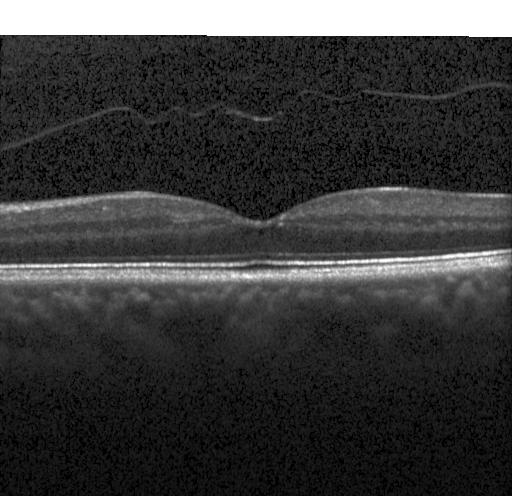 Horizontal scan through the fovea. Retinal OCT B-scan. Heidelberg Spectralis. Spectral-domain OCT
No choroidal neovascularization, no diabetic macular edema, and no drusen.